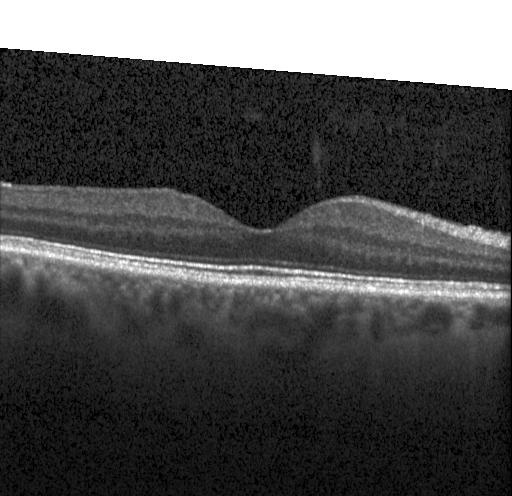
OCT B-scan. Acquired on a Heidelberg Spectralis. Macular scan. SD-OCT.
The scan shows no choroidal neovascularization, diabetic macular edema, or drusen.